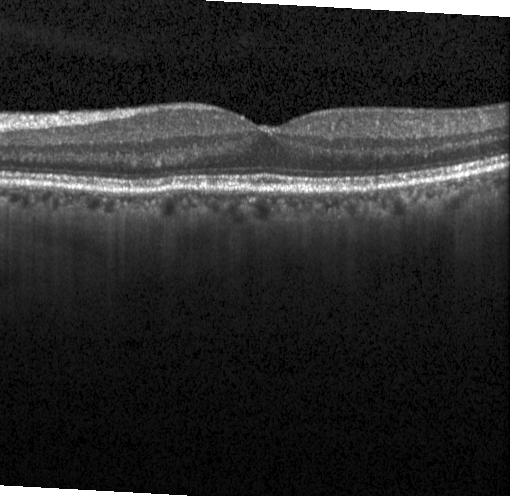
Retinal OCT cross-section
This B-scan demonstrates no choroidal neovascularization, diabetic macular edema, or drusen.